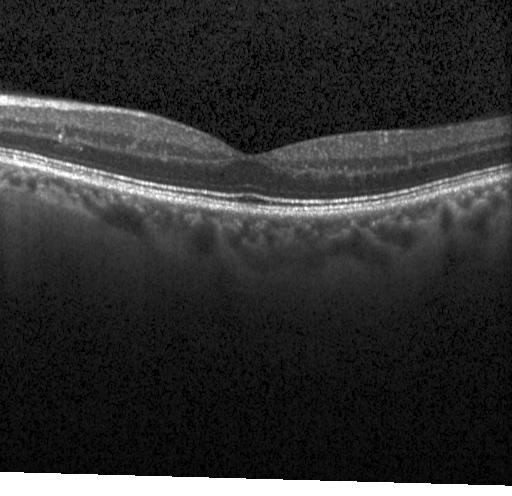

Horizontal scan through the fovea; spectral-domain OCT; retinal OCT cross-section. Dx: neither choroidal neovascularization, diabetic macular edema, nor drusen.